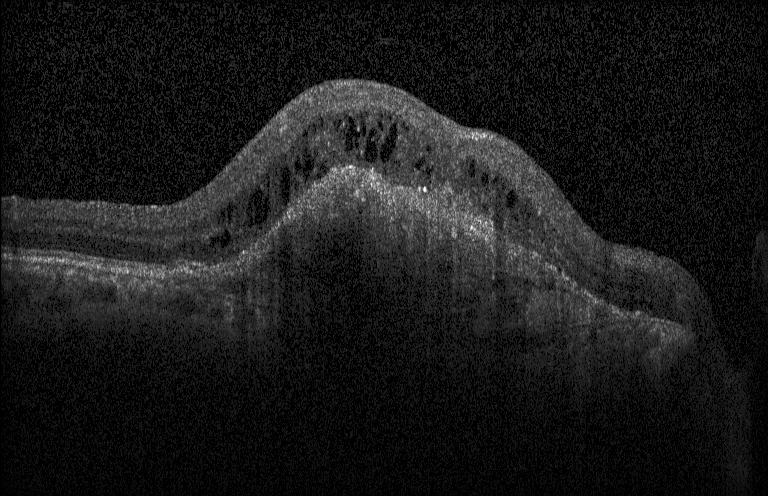 Choroidal neovascularization (CNV).